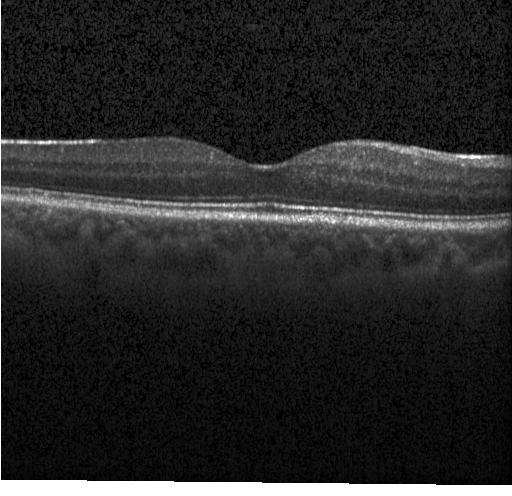 Finding: no choroidal neovascularization, diabetic macular edema, or drusen.